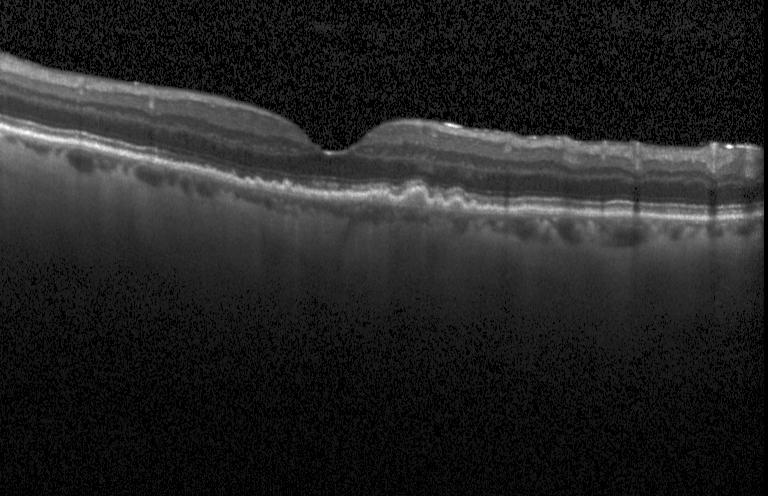 OCT finding: drusen.